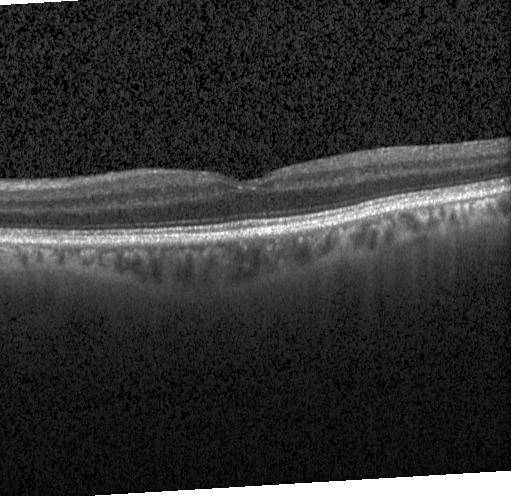 Spectral-domain OCT B-scan: no evidence of CNV, DME, or drusen.